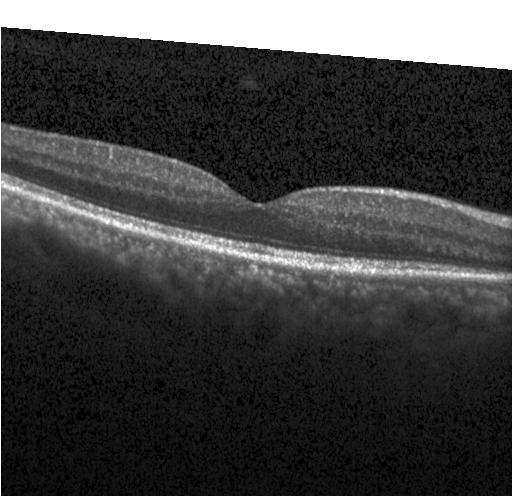
Retinal OCT B-scan, spectral-domain optical coherence tomography, centered on the fovea.
Impression: no evidence of CNV, DME, or drusen.